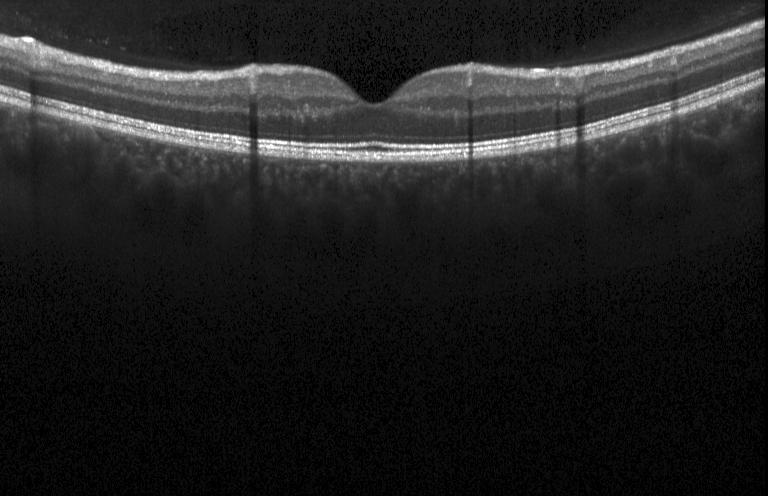

Fovea-centered · optical coherence tomography scan
Impression: no evidence of CNV, DME, or drusen.